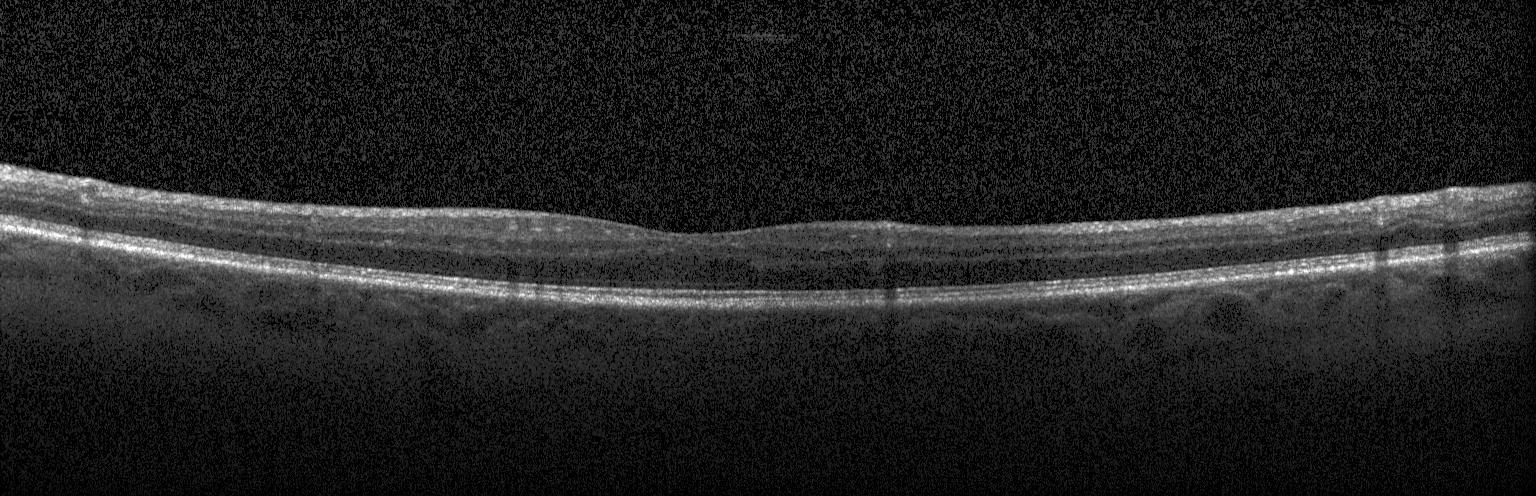

Fovea-centered. Retinal OCT cross-section
The scan shows no choroidal neovascularization, diabetic macular edema, or drusen.